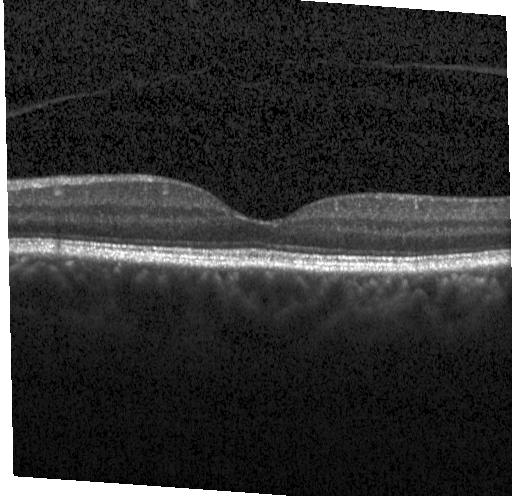 No evidence of choroidal neovascularization, diabetic macular edema, or drusen.